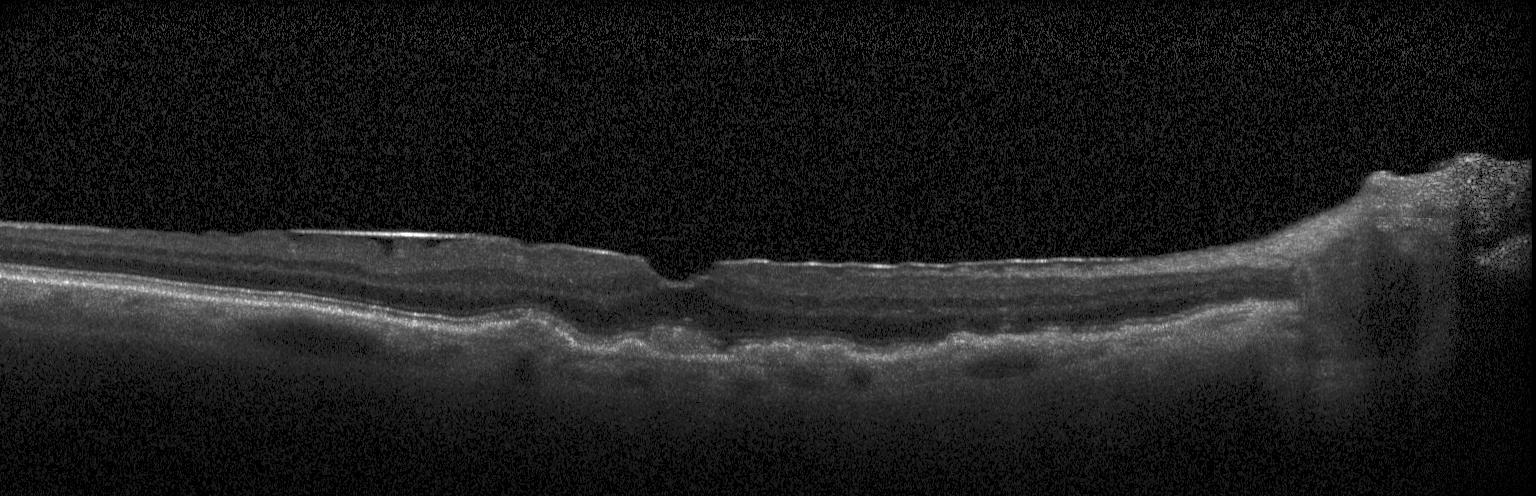
Diagnosis: sub-RPE drusenoid deposits.